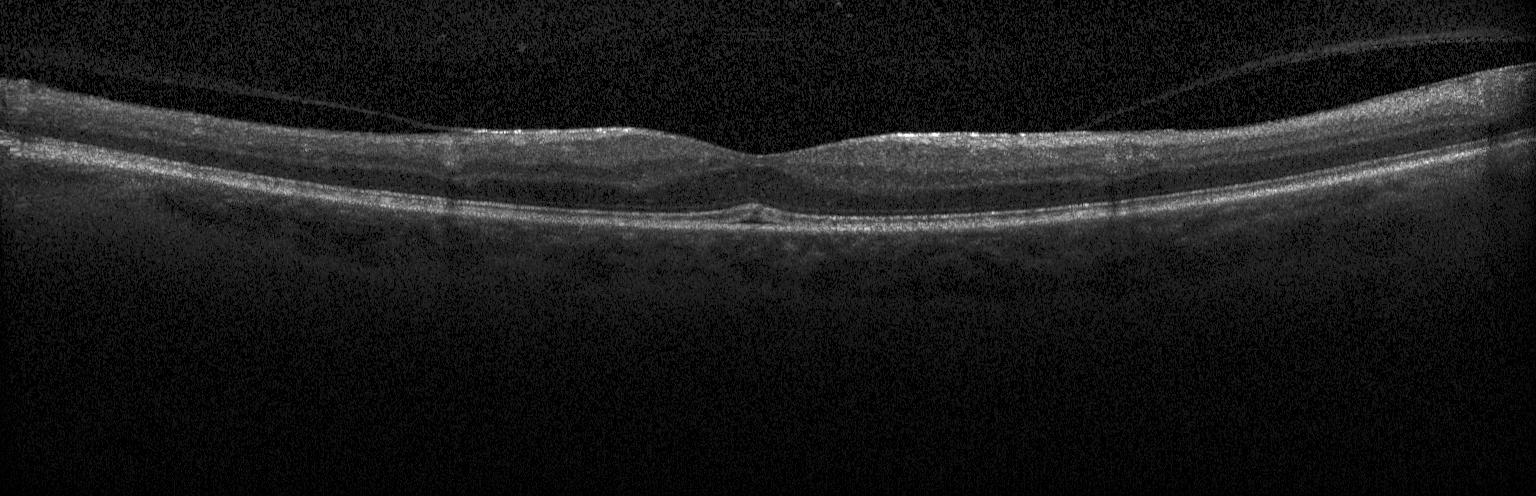

Optical coherence tomography B-scan. SD-OCT. Heidelberg Spectralis OCT system. Fovea-centered
Dx: no choroidal neovascularization, no diabetic macular edema, and no drusen.